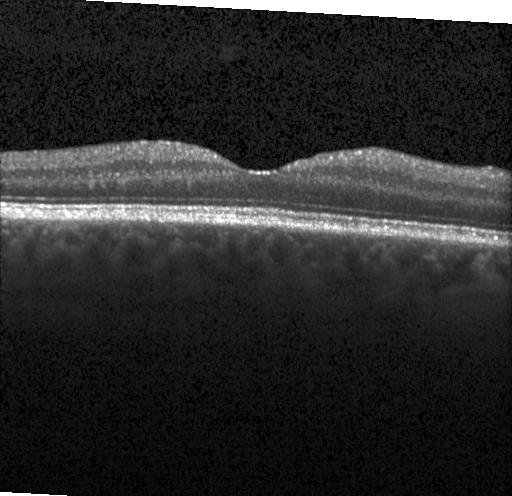 Heidelberg Spectralis; optical coherence tomography scan; horizontal scan through the fovea. Diagnosis: neither choroidal neovascularization, diabetic macular edema, nor drusen.